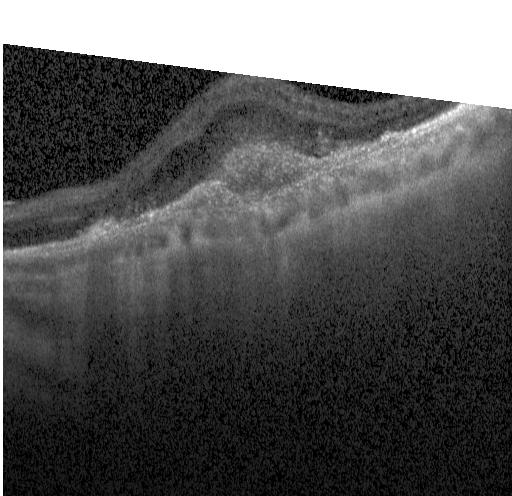

Macular scan. OCT B-scan. SD-OCT. Heidelberg Spectralis OCT system
Macular OCT: choroidal neovascularization.